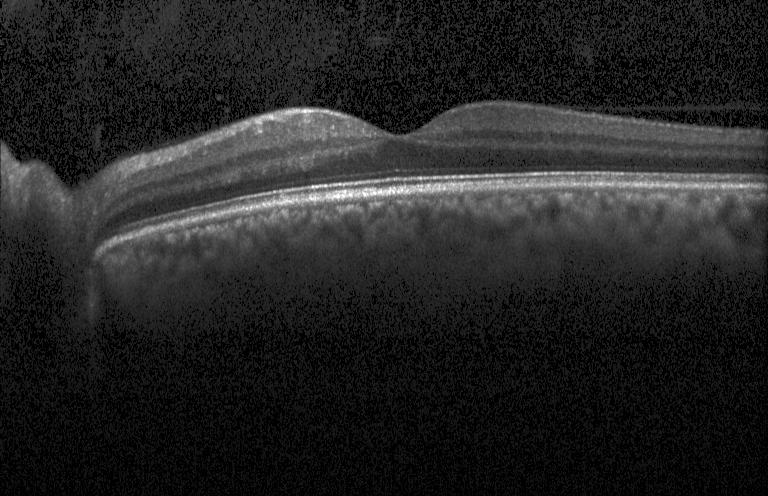

Centered on the fovea. OCT line scan. Instrument: Heidelberg Spectralis — No CNV, no DME, and no drusen.